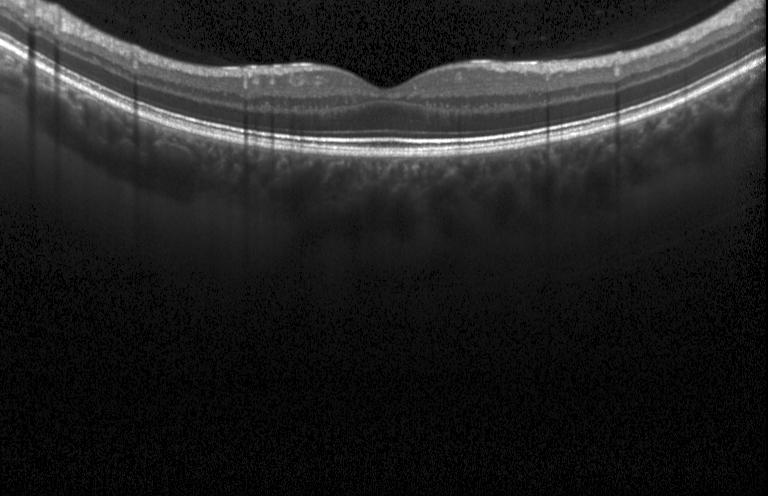 Retinal OCT B-scan, macular scan, Heidelberg Spectralis, SD-OCT — Dx: neither CNV, DME, nor drusen.